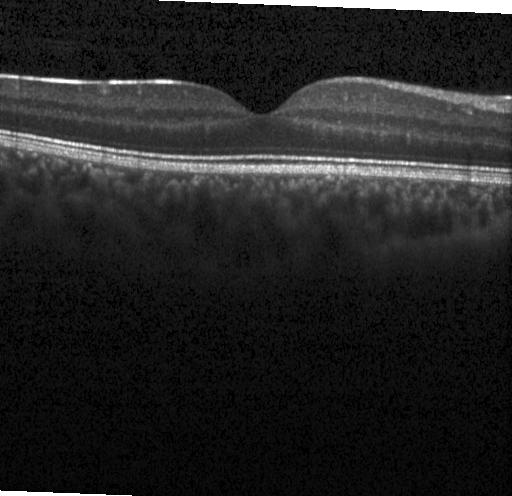

Finding: no evidence of choroidal neovascularization, diabetic macular edema, or drusen.